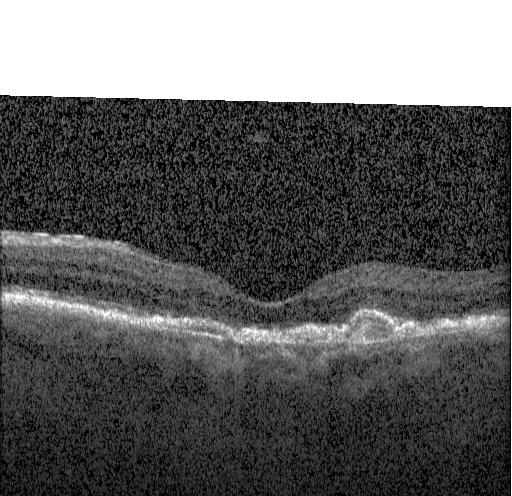
OCT line scan. SD-OCT. Heidelberg Spectralis. Diagnosis: choroidal neovascularization.